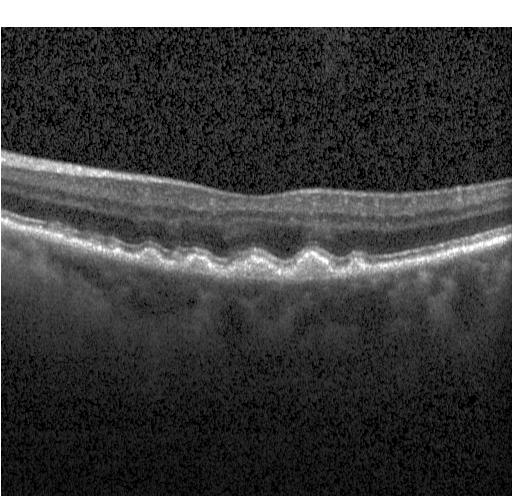 Retinal OCT cross-section. Centered on the fovea. Heidelberg Spectralis OCT system — The scan shows multiple drusen.